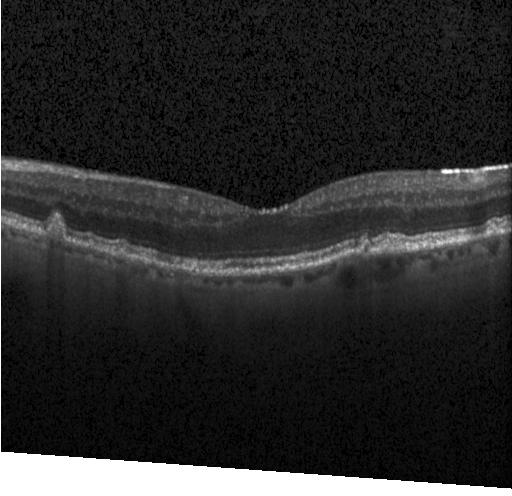

OCT finding: sub-RPE drusenoid deposits.